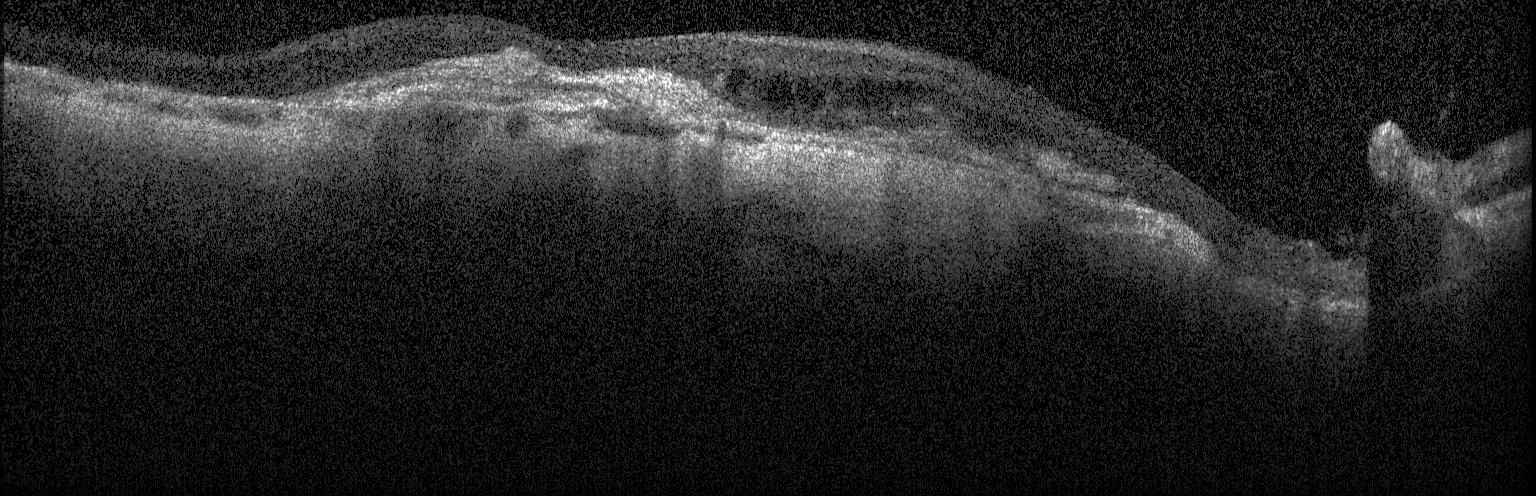

OCT B-scan showing choroidal neovascularization (CNV).